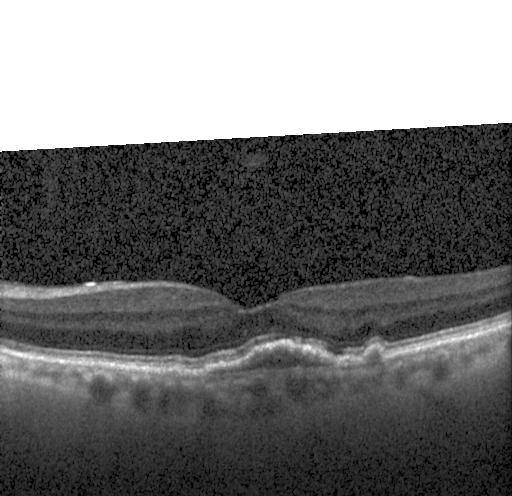
Fovea-centered, acquired on a Heidelberg Spectralis, retinal OCT B-scan
Finding: a choroidal neovascular membrane.